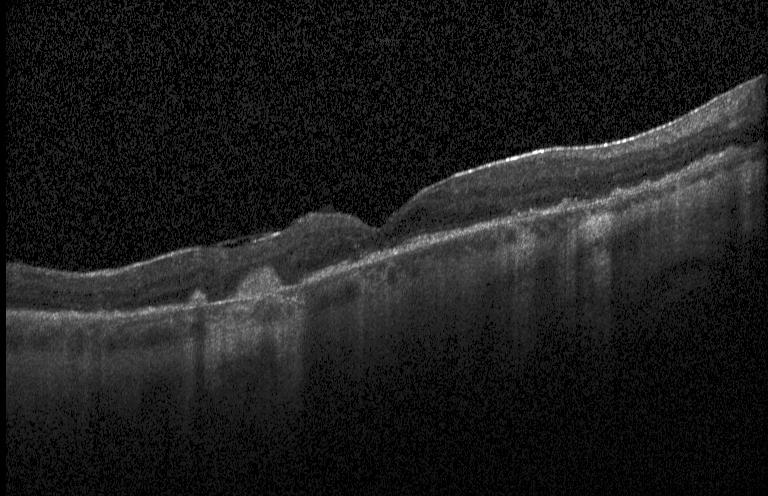
OCT B-scan showing a choroidal neovascular membrane.